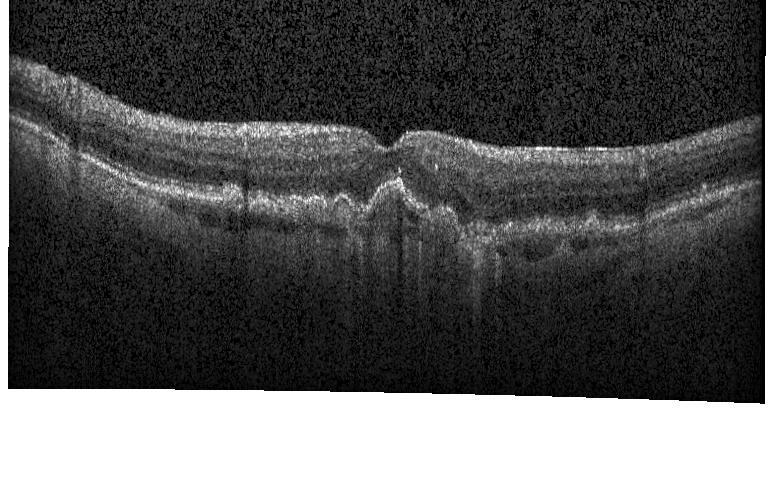

Macular scan, OCT line scan.
The scan shows choroidal neovascularization.